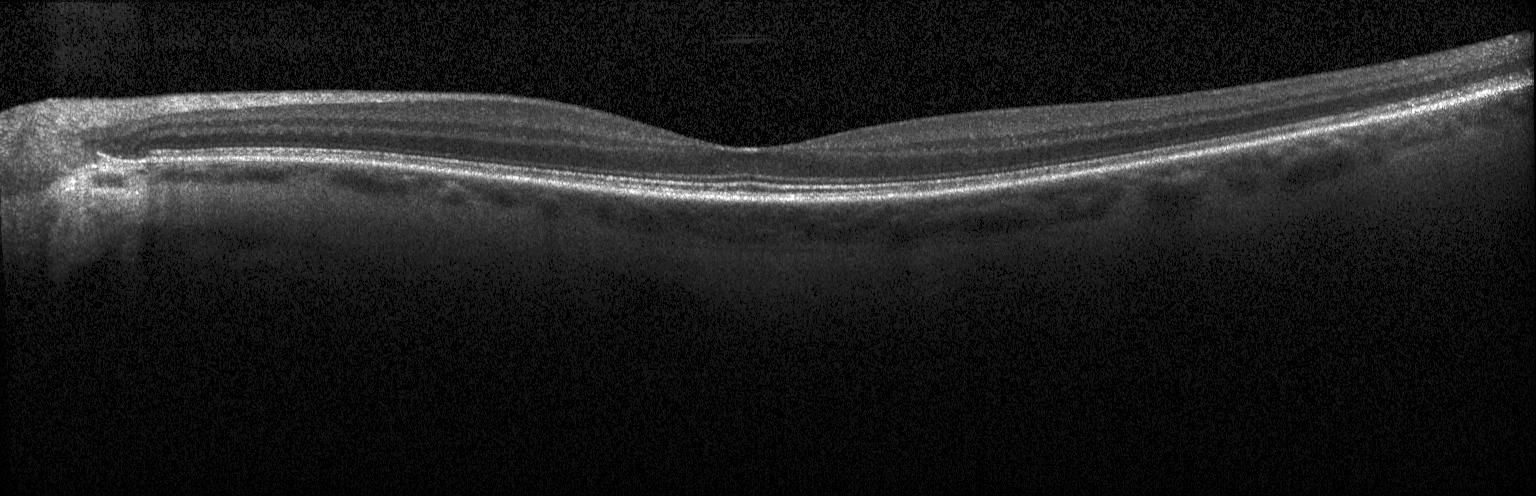

OCT line scan — Diagnosis: no choroidal neovascularization, diabetic macular edema, or drusen.